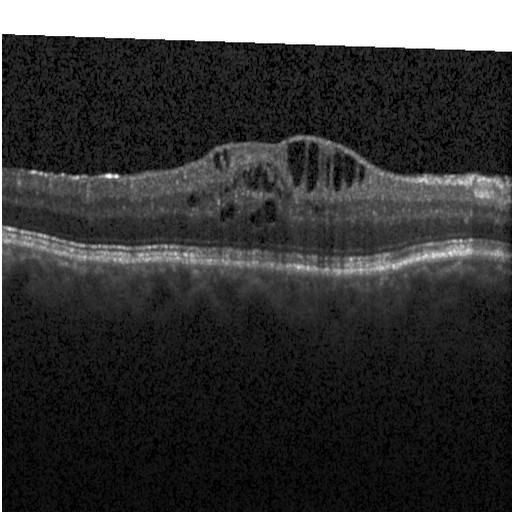 Impression: diabetic macular edema.